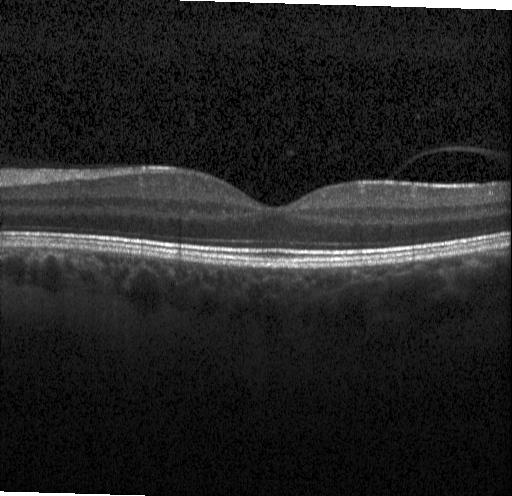 Heidelberg Spectralis; spectral-domain optical coherence tomography; retinal OCT B-scan; centered on the fovea. Dx: no evidence of choroidal neovascularization, diabetic macular edema, or drusen.